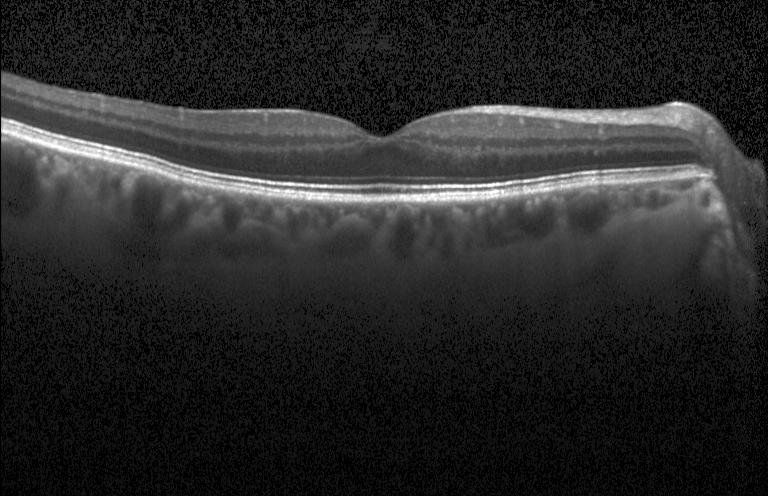 OCT B-scan.
Diagnosis: neither choroidal neovascularization, diabetic macular edema, nor drusen.